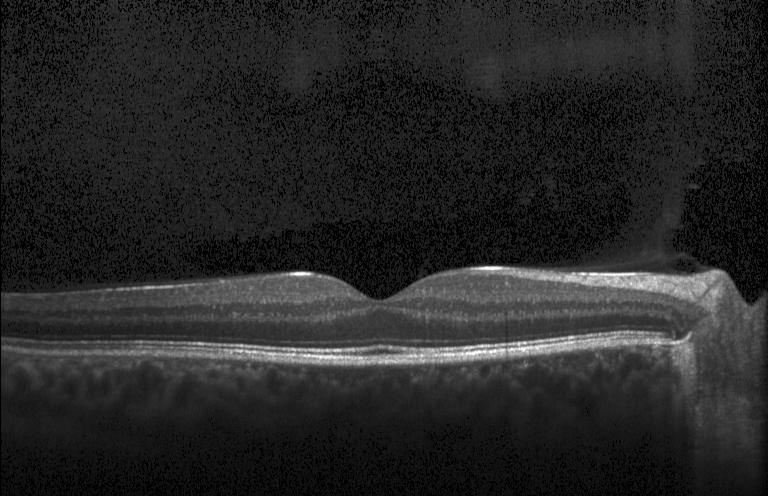 OCT finding: no choroidal neovascularization, diabetic macular edema, or drusen.